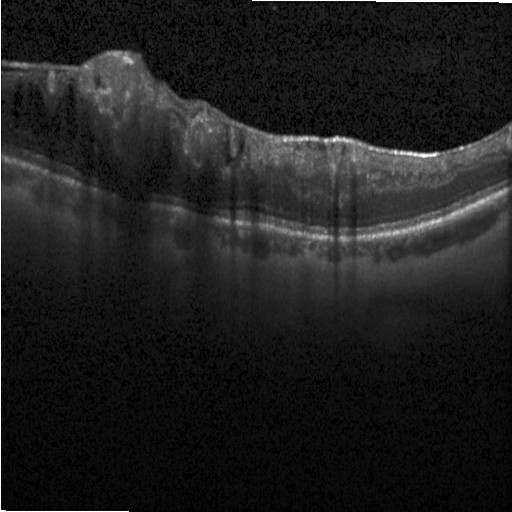
OCT line scan. Fovea-centered. Spectral-domain optical coherence tomography. Instrument: Heidelberg Spectralis
Diagnosis: diabetic macular edema (DME).